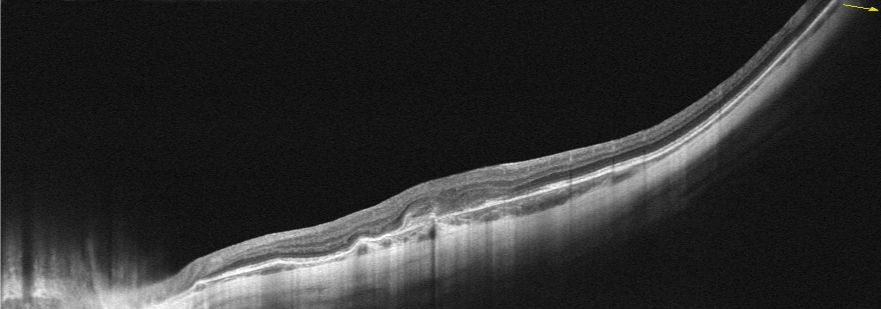

Acquired on an Optovue Avanti RTVue XR · OCT line scan · fovea-centered.
Diagnosis: age-related macular degeneration (AMD).